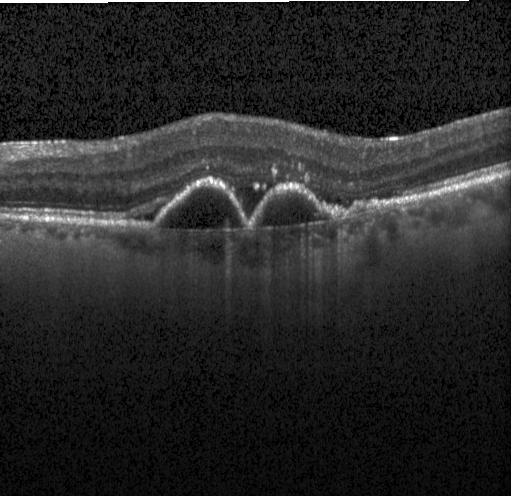
Retinal OCT cross-section showing CNV.